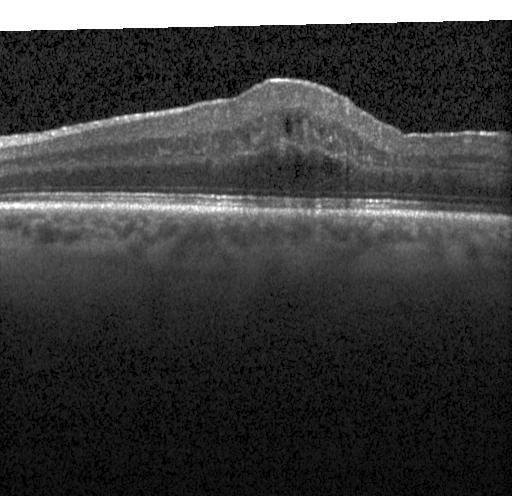
Optical coherence tomography scan — Diagnosis: DME.